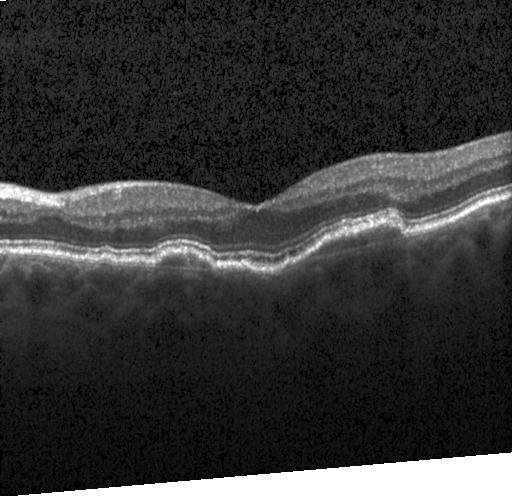
OCT B-scan.
CNV.